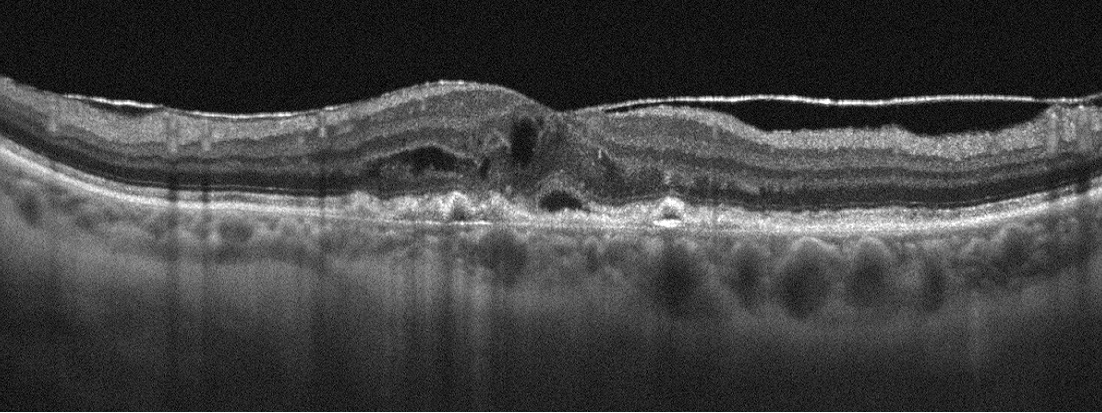 Dx: age-related macular degeneration.